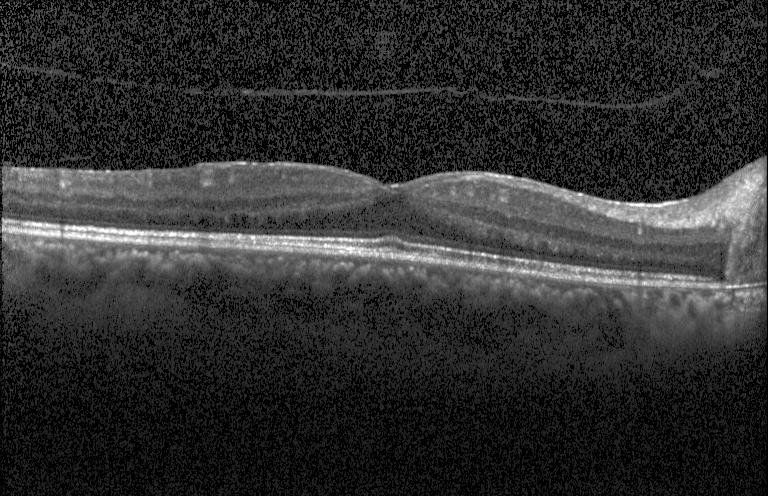
No choroidal neovascularization, diabetic macular edema, or drusen.